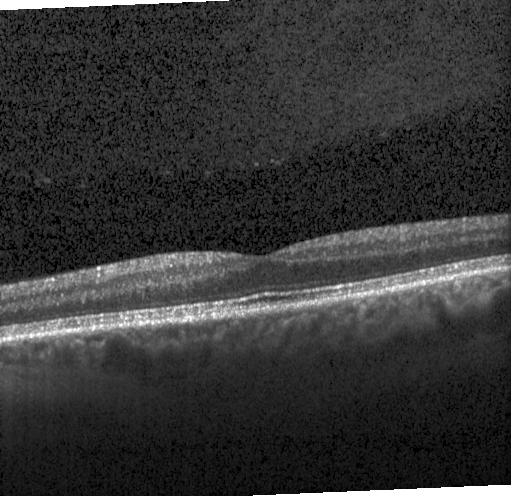

Retinal OCT cross-section; Heidelberg Spectralis OCT system; horizontal scan through the fovea; spectral-domain optical coherence tomography — Assessment: no choroidal neovascularization, no diabetic macular edema, and no drusen.